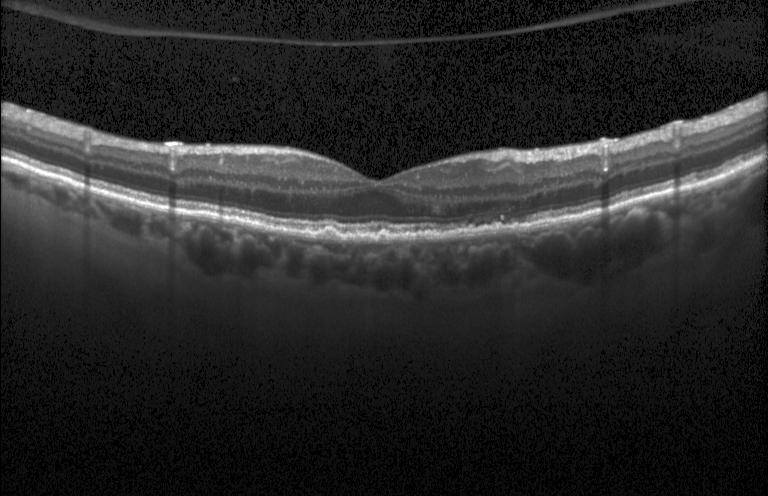
OCT B-scan, Heidelberg Spectralis OCT system. OCT finding: multiple drusen.